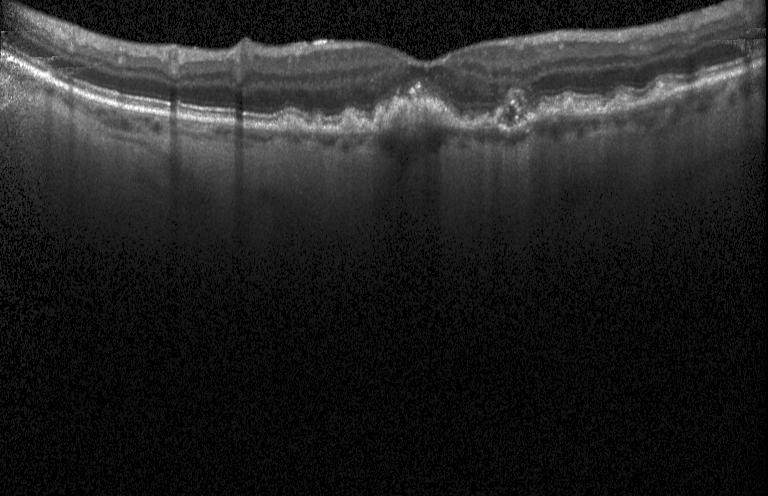

OCT B-scan showing a choroidal neovascular membrane.